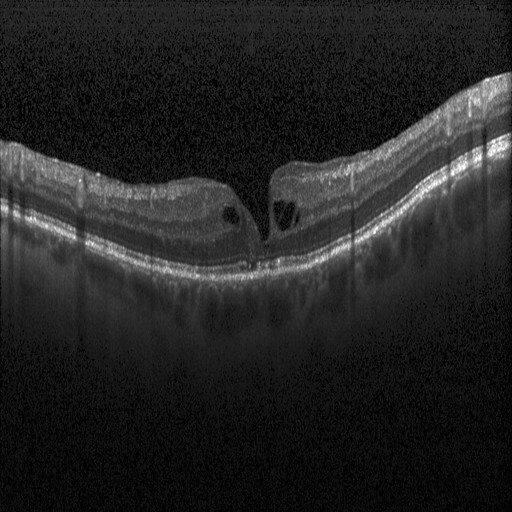
Through the macula; OCT B-scan; acquired on a Heidelberg Spectralis.
DME.